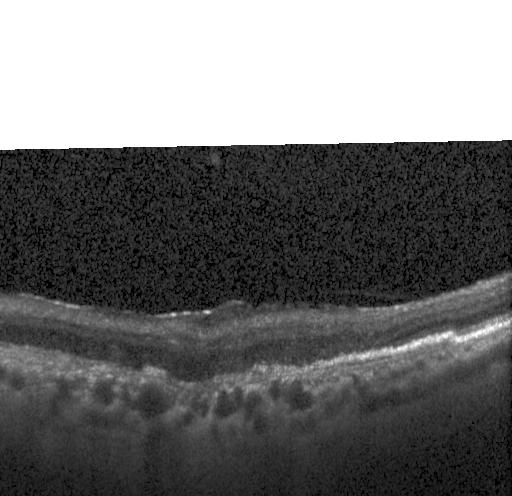

Optical coherence tomography scan. Impression: a choroidal neovascular membrane.